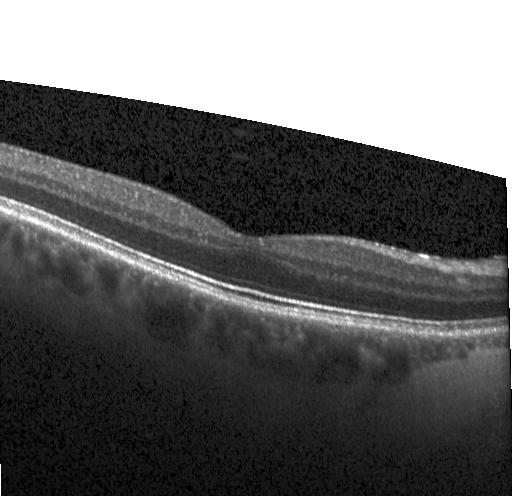

OCT line scan · spectral-domain optical coherence tomography · fovea-centered · Heidelberg Spectralis OCT system — This B-scan demonstrates no evidence of choroidal neovascularization, diabetic macular edema, or drusen.